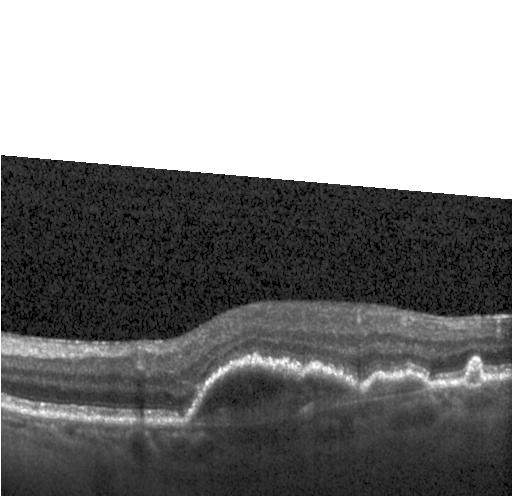 Spectral-domain optical coherence tomography. Instrument: Heidelberg Spectralis. Optical coherence tomography B-scan — Assessment: choroidal neovascularization.